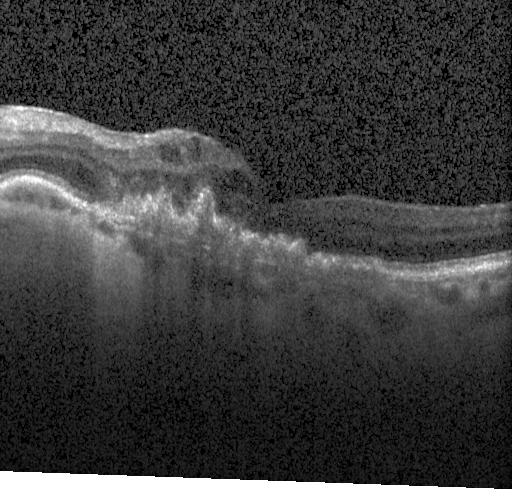

Retinal OCT cross-section — Finding: choroidal neovascularization (CNV).